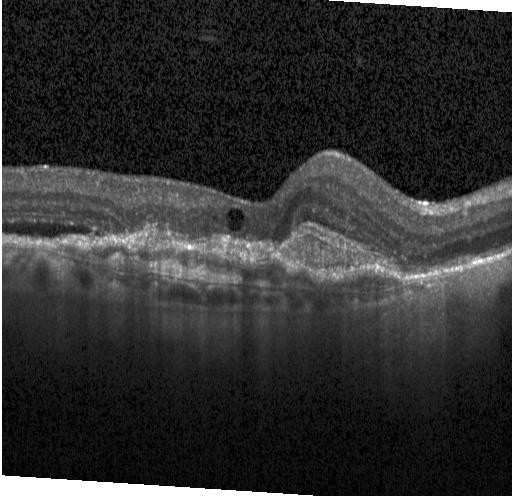
Acquired on a Heidelberg Spectralis · SD-OCT · through the macula · retinal OCT cross-section. Assessment: CNV.